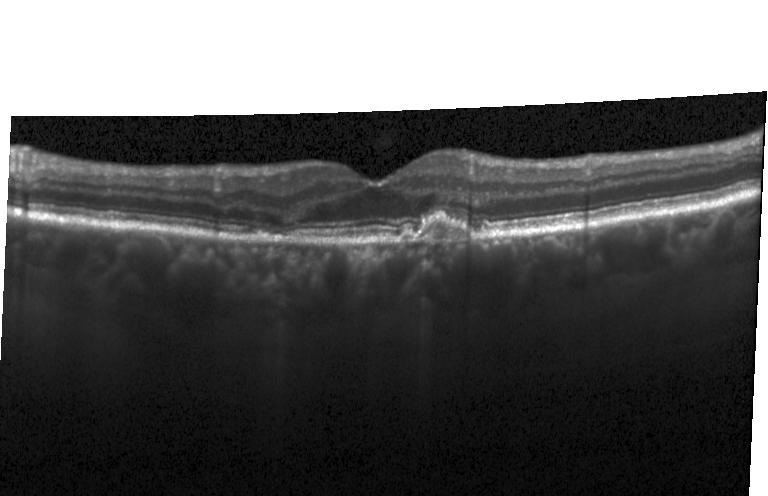

SD-OCT. OCT B-scan. Heidelberg Spectralis OCT system. Centered on the fovea
Finding: a choroidal neovascular membrane.